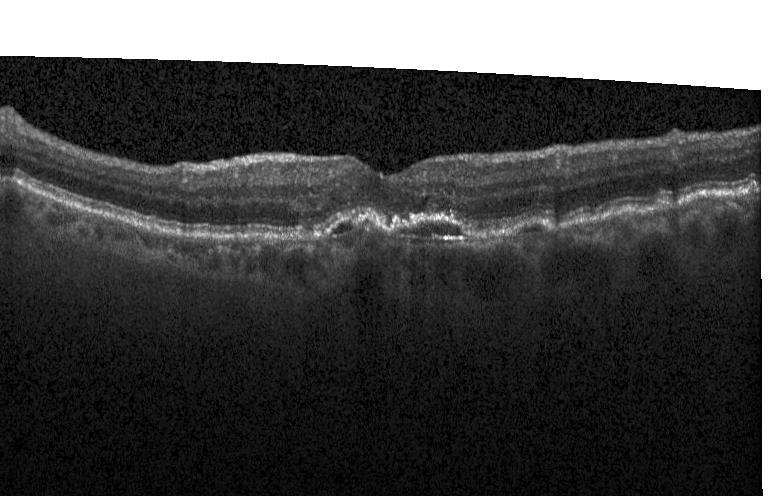
The scan shows a choroidal neovascular membrane.